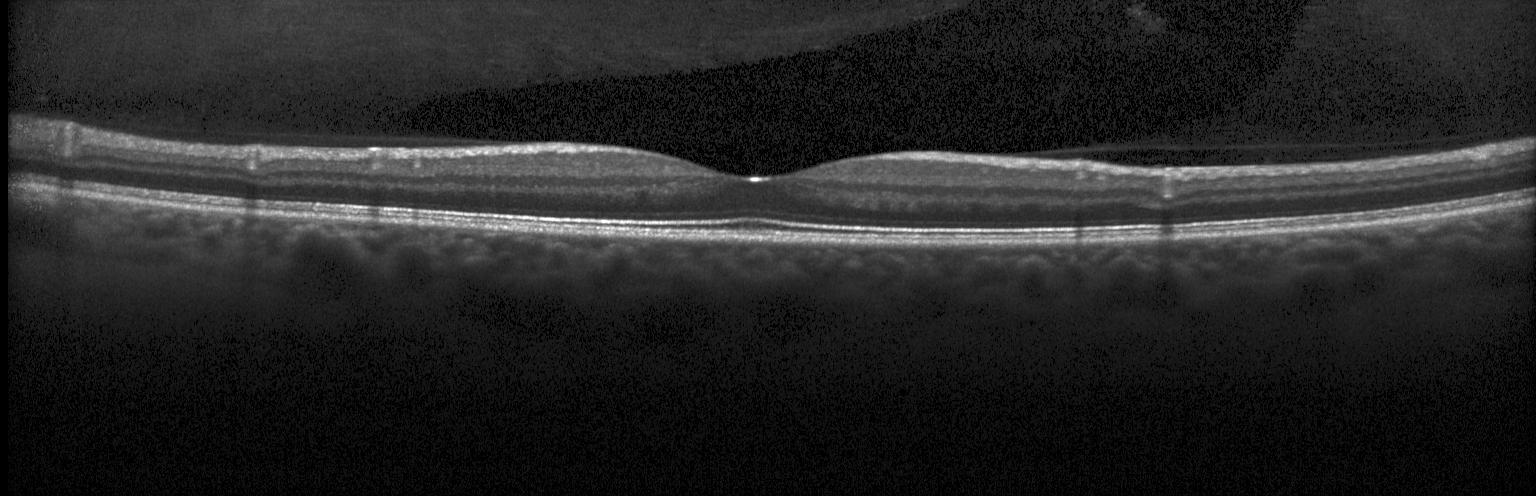

SD-OCT; Heidelberg Spectralis; OCT line scan; horizontal scan through the fovea — Finding: no choroidal neovascularization, no diabetic macular edema, and no drusen.